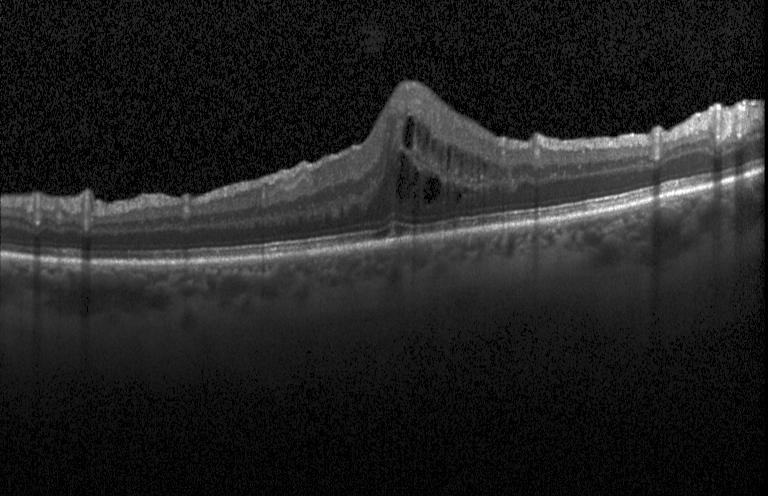 Optical coherence tomography scan. Diagnosis: DME.